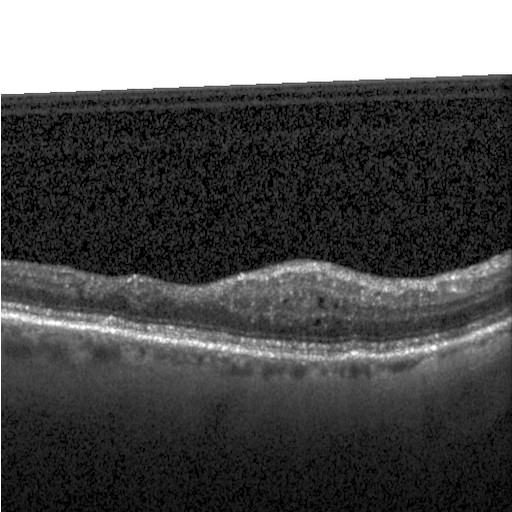
OCT finding: diabetic macular edema (DME).